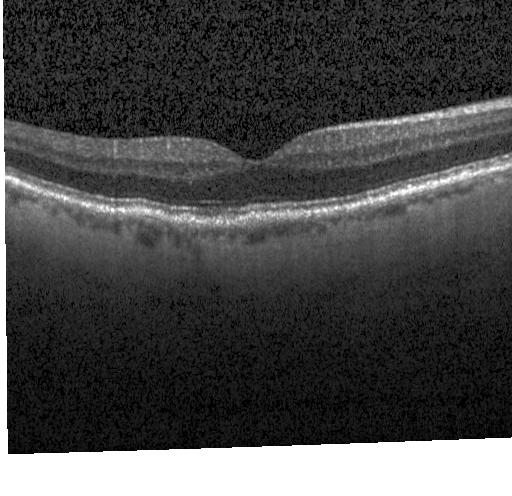

Retinal OCT cross-section showing neither choroidal neovascularization, diabetic macular edema, nor drusen.